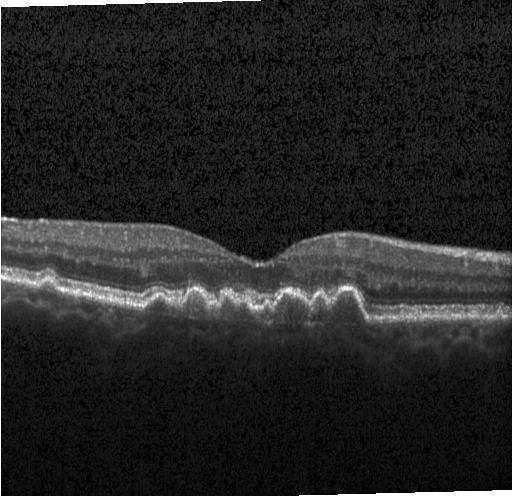
Spectral-domain OCT; OCT B-scan; centered on the fovea.
Impression: multiple drusen.